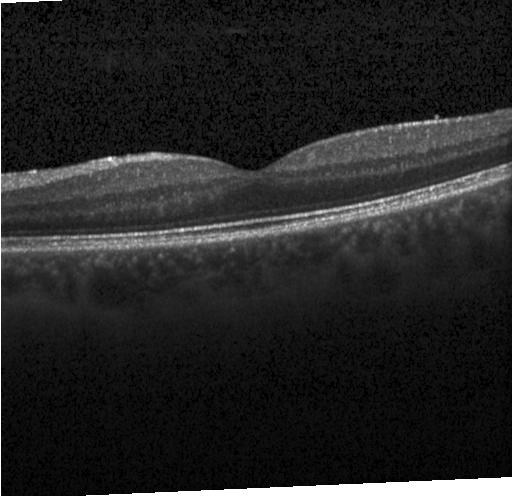
Fovea-centered; optical coherence tomography scan. Finding: no CNV, DME, or drusen.